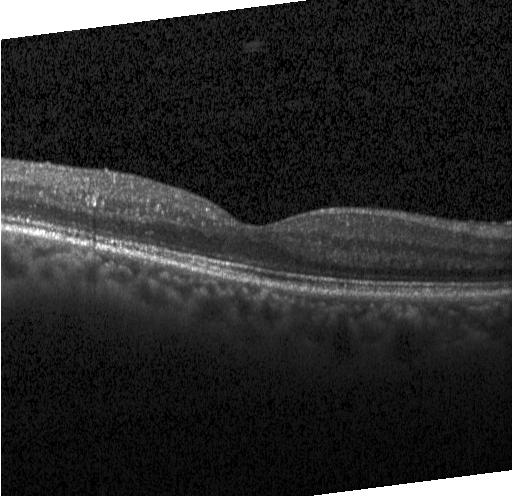

Diagnosis: neither choroidal neovascularization, diabetic macular edema, nor drusen.